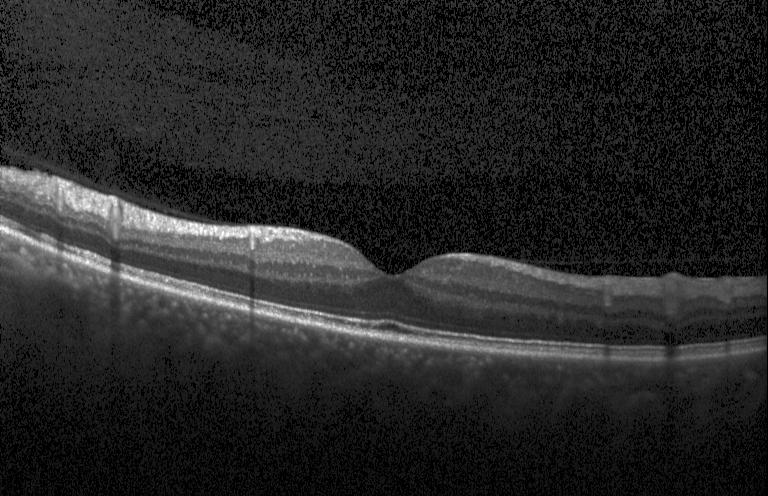 Impression: no CNV, DME, or drusen.